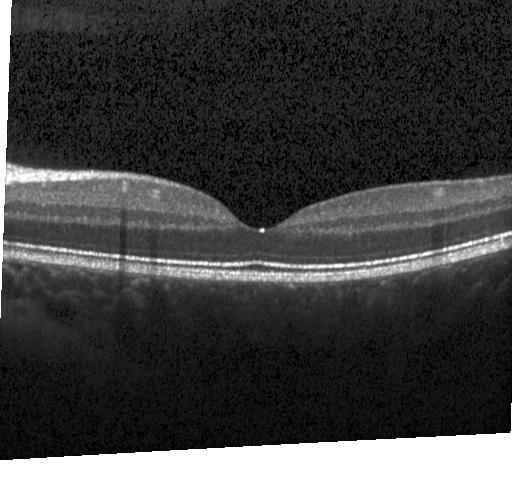

Macular scan; spectral-domain OCT; Heidelberg Spectralis; OCT line scan. Diagnosis: neither choroidal neovascularization, diabetic macular edema, nor drusen.